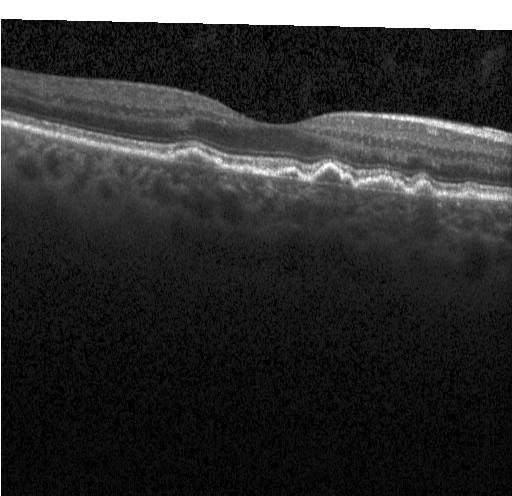
Macular OCT: multiple drusen.